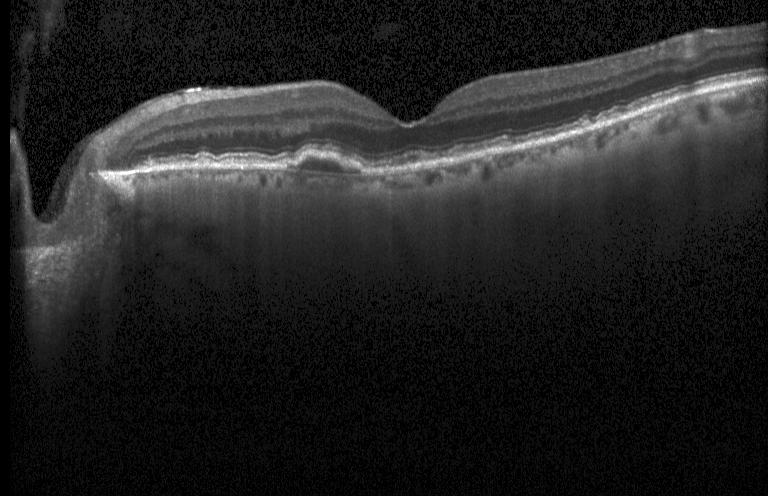

Spectral-domain OCT; macular scan; instrument: Heidelberg Spectralis; OCT B-scan — Finding: a choroidal neovascular membrane.